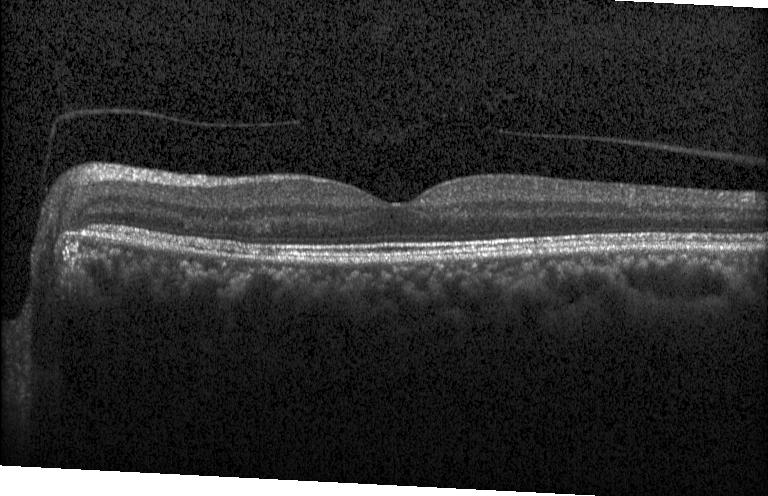

Macular OCT demonstrating neither choroidal neovascularization, diabetic macular edema, nor drusen.